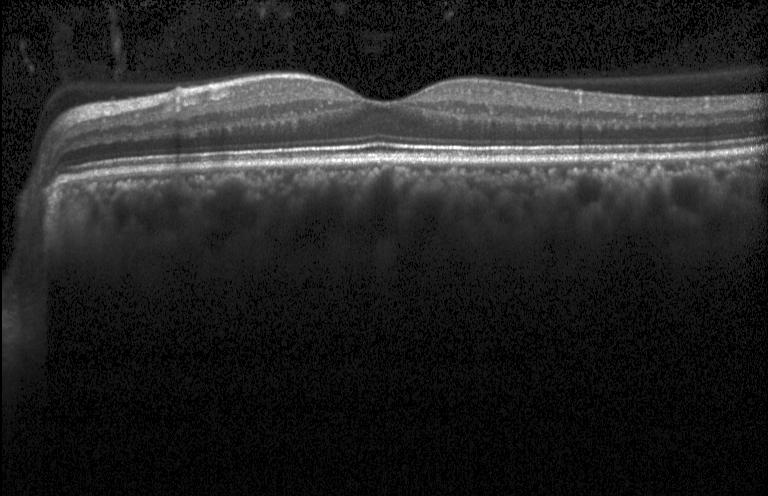

Spectral-domain OCT B-scan: no CNV, DME, or drusen.